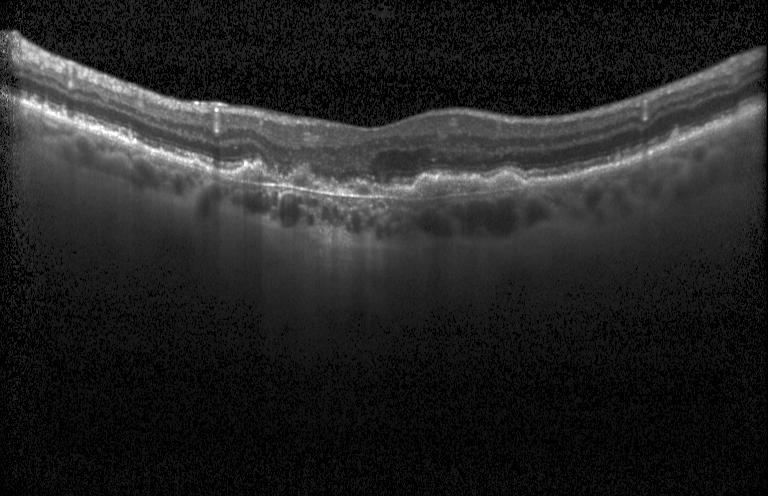
Impression: choroidal neovascularization.